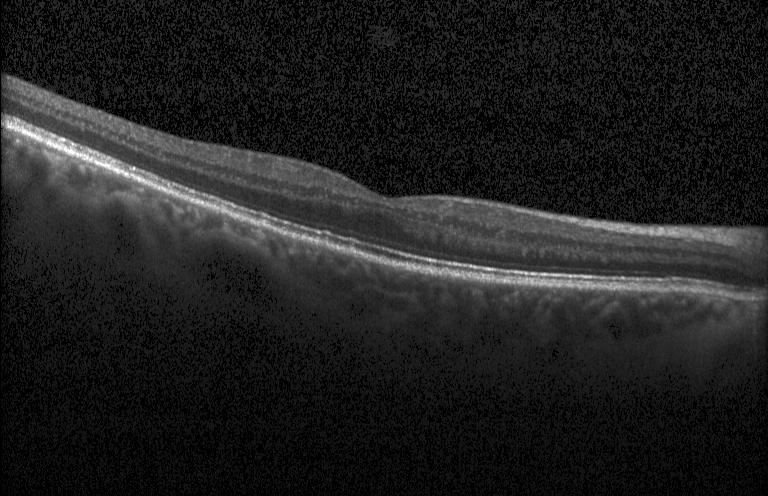
Optical coherence tomography B-scan — Assessment: neither choroidal neovascularization, diabetic macular edema, nor drusen.